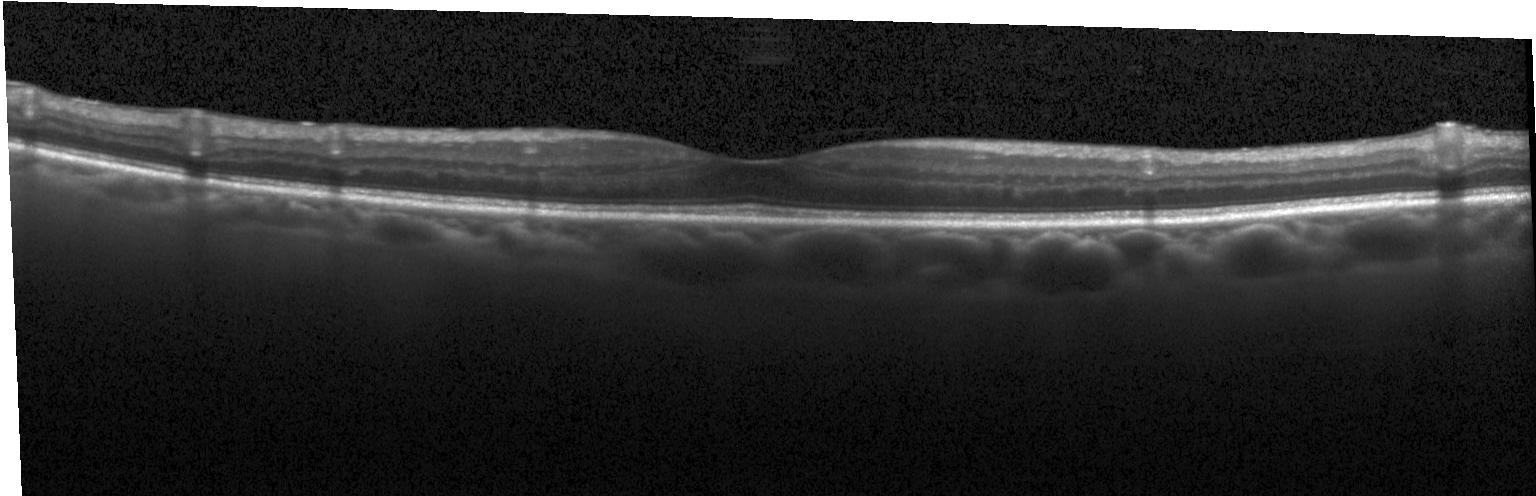 Finding: neither CNV, DME, nor drusen.